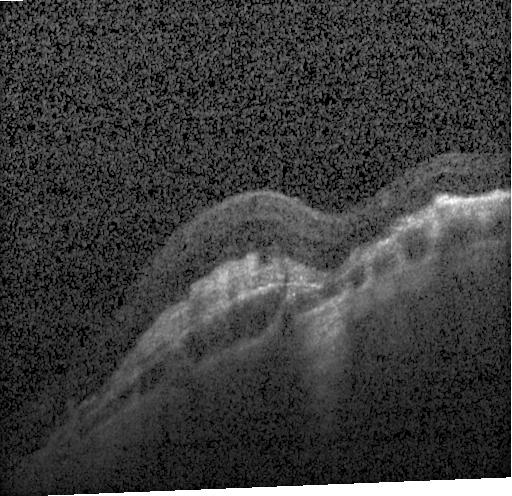 Macular OCT: choroidal neovascularization.